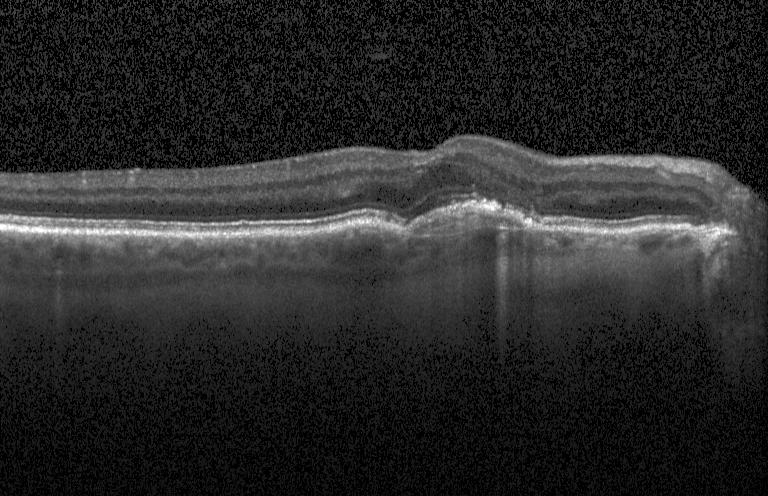

OCT finding: choroidal neovascularization (CNV).